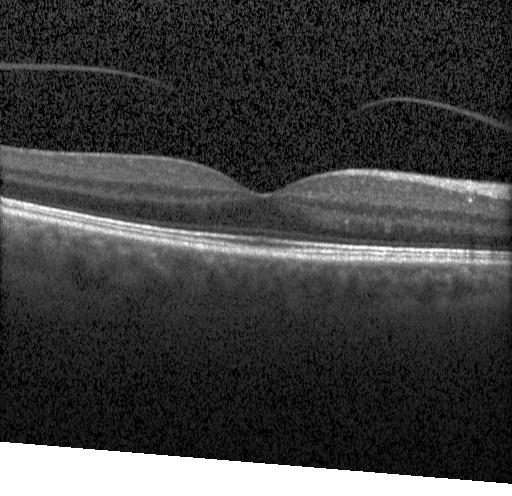 Optical coherence tomography B-scan
Impression: no CNV, no DME, and no drusen.